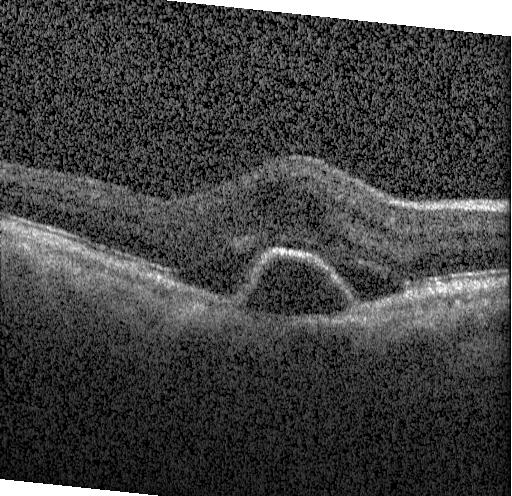
OCT line scan, fovea-centered, SD-OCT. Dx: choroidal neovascularization.